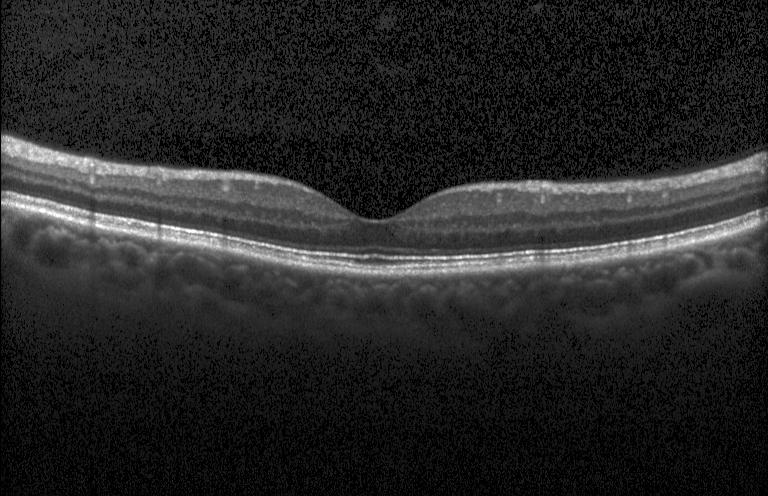

OCT B-scan showing no evidence of choroidal neovascularization, diabetic macular edema, or drusen.